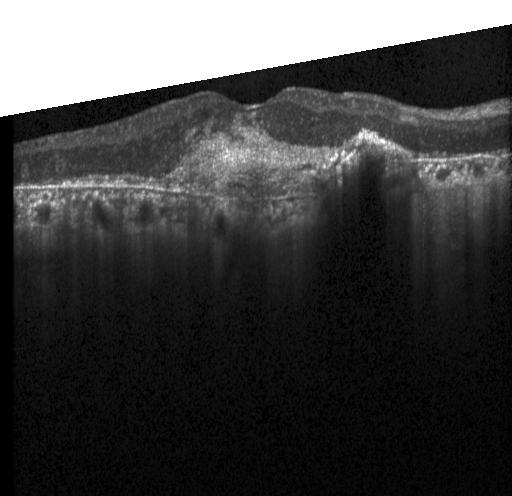

OCT B-scan — Macular OCT: CNV.